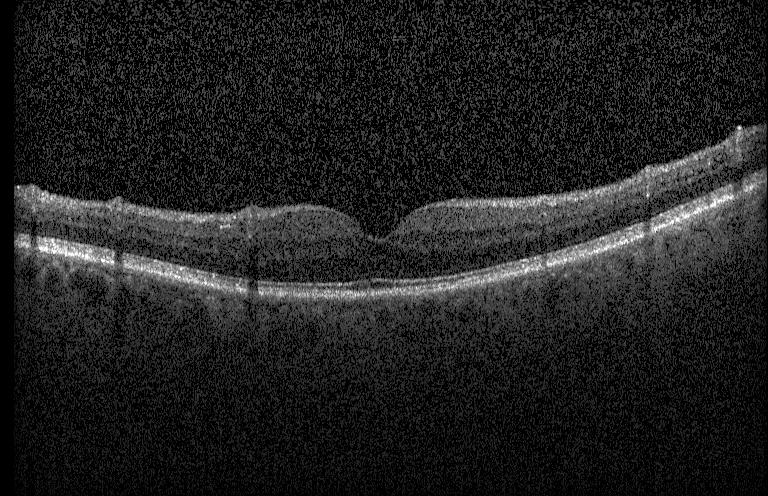
SD-OCT; Heidelberg Spectralis OCT system; macular scan; OCT B-scan. Diagnosis: no choroidal neovascularization, no diabetic macular edema, and no drusen.